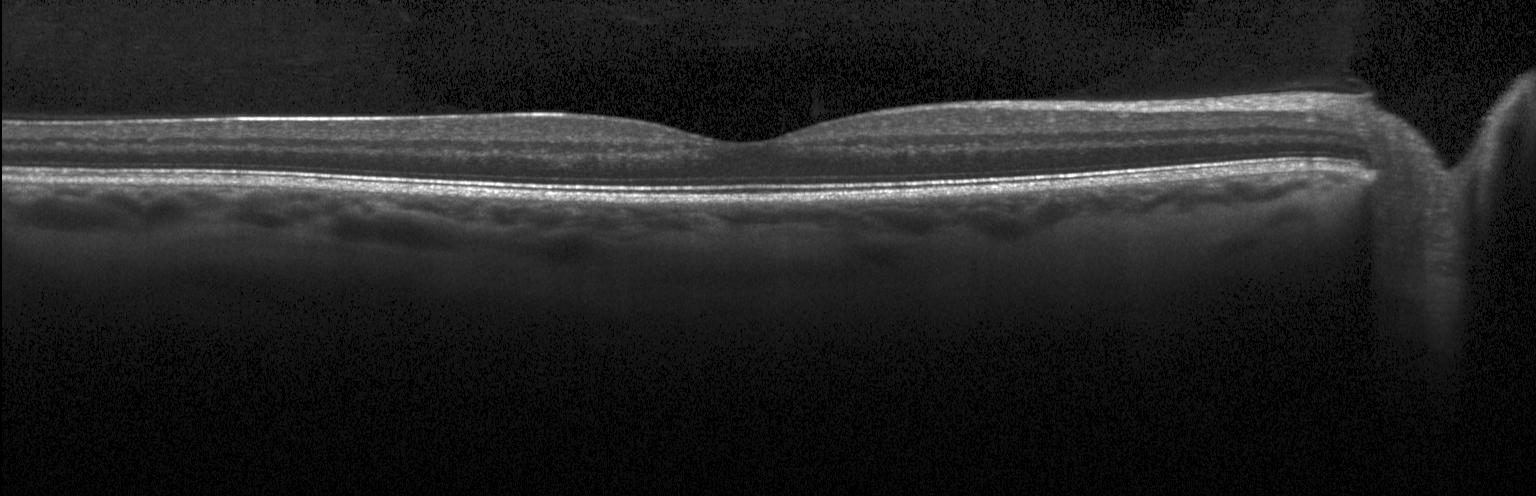
Macular OCT: no choroidal neovascularization, diabetic macular edema, or drusen.